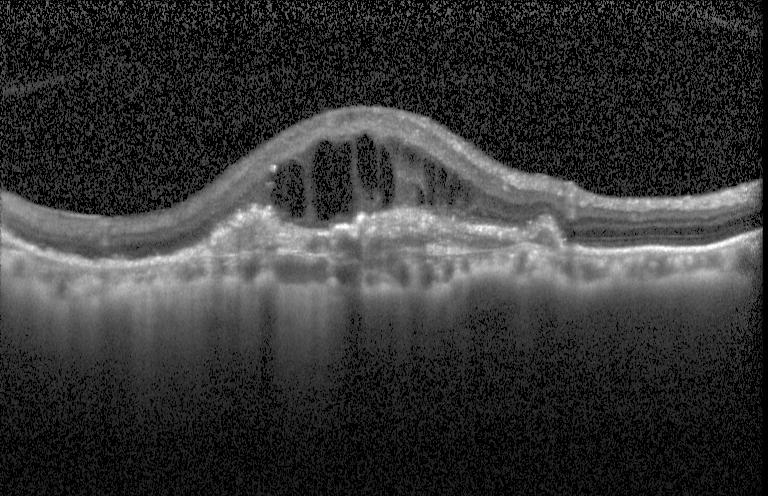

Dx: a choroidal neovascular membrane.